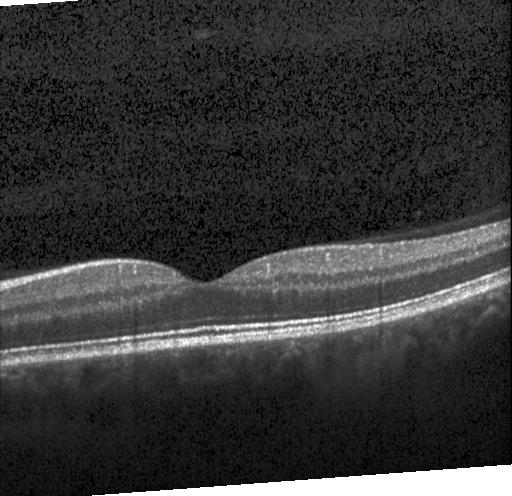 OCT line scan, through the macula.
OCT finding: no evidence of choroidal neovascularization, diabetic macular edema, or drusen.